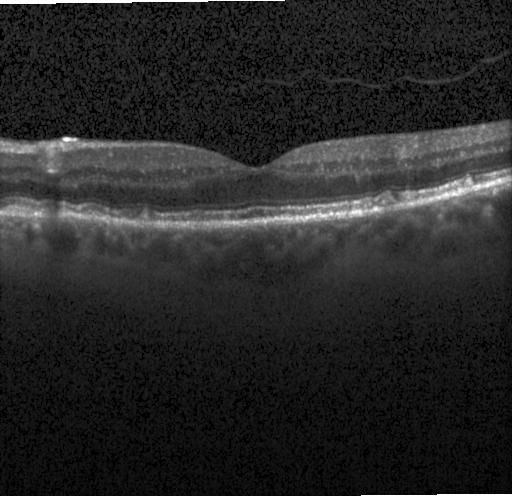
Macular scan · optical coherence tomography scan. Diagnosis: drusen.